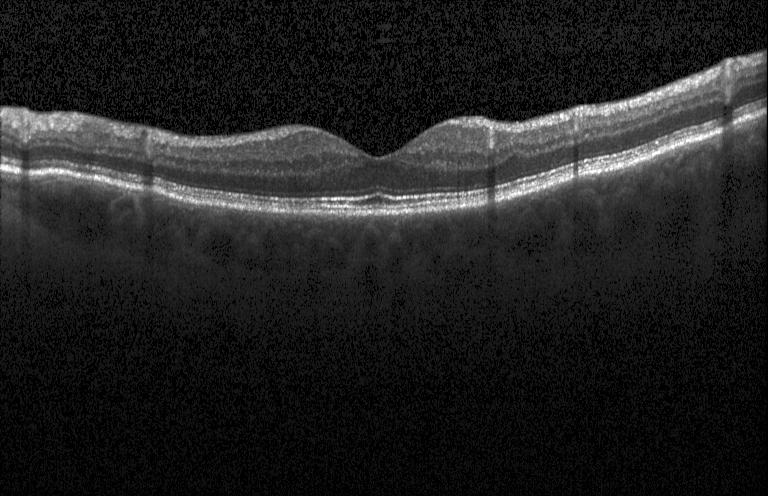 Impression: neither CNV, DME, nor drusen.